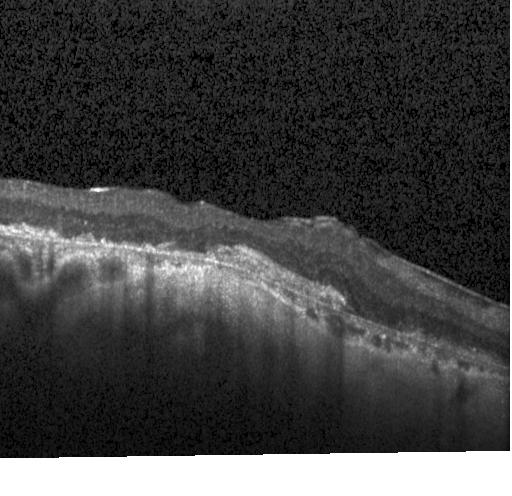 Through the macula. Retinal OCT B-scan. Finding: CNV.